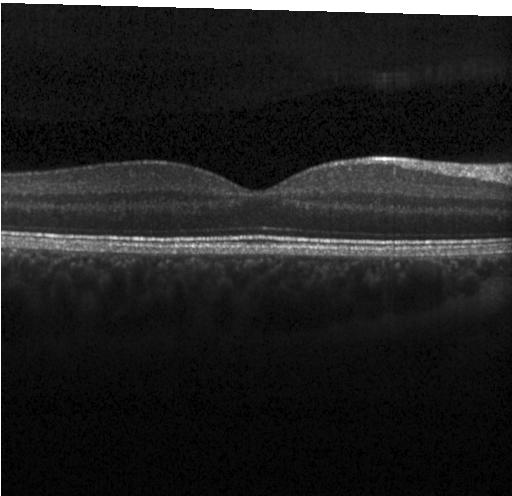
Spectral-domain OCT B-scan: no evidence of CNV, DME, or drusen.